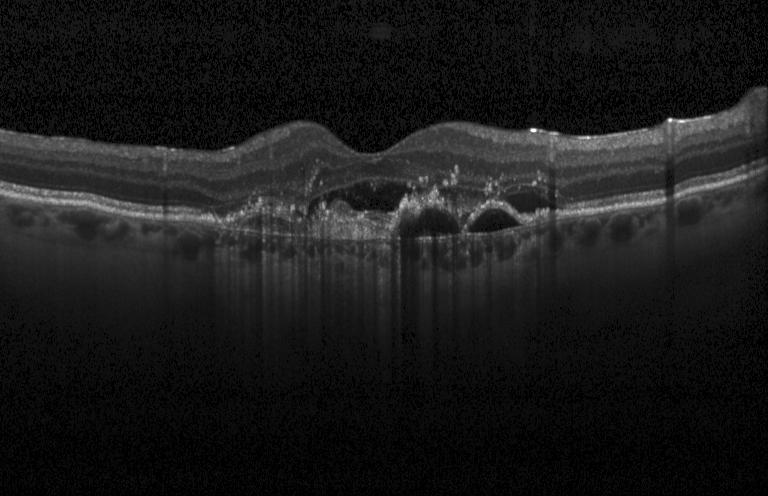
Heidelberg Spectralis OCT system, macular scan, spectral-domain optical coherence tomography, optical coherence tomography B-scan. Finding: a choroidal neovascular membrane.